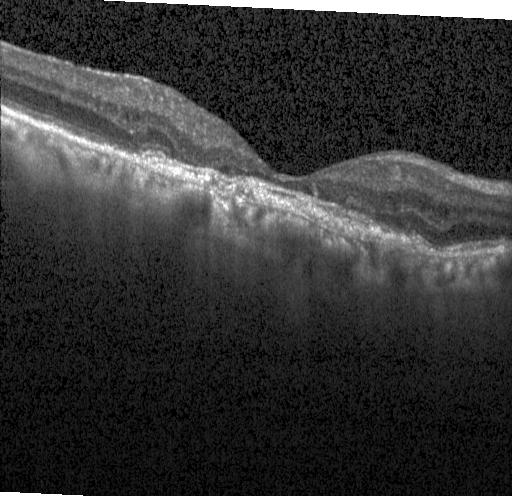

Impression: choroidal neovascularization (CNV).